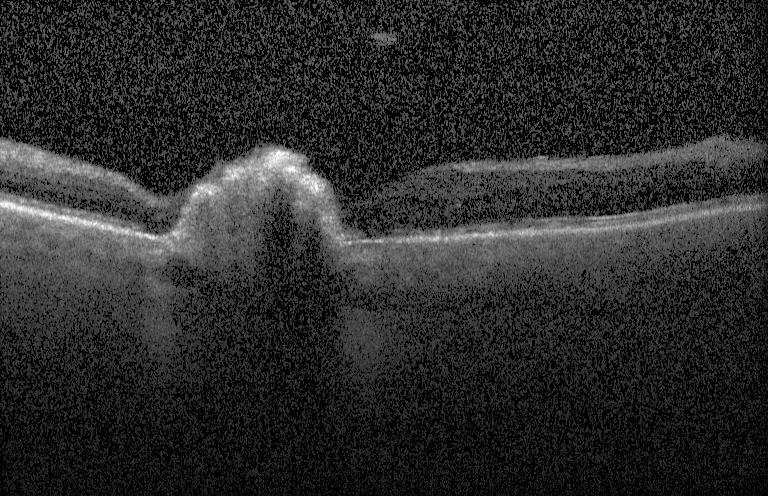

Macular OCT demonstrating choroidal neovascularization.